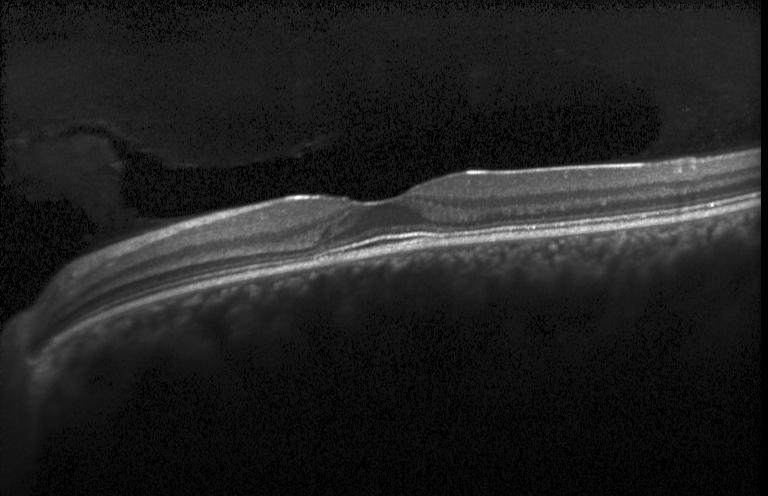
SD-OCT. OCT line scan — Impression: no choroidal neovascularization, diabetic macular edema, or drusen.